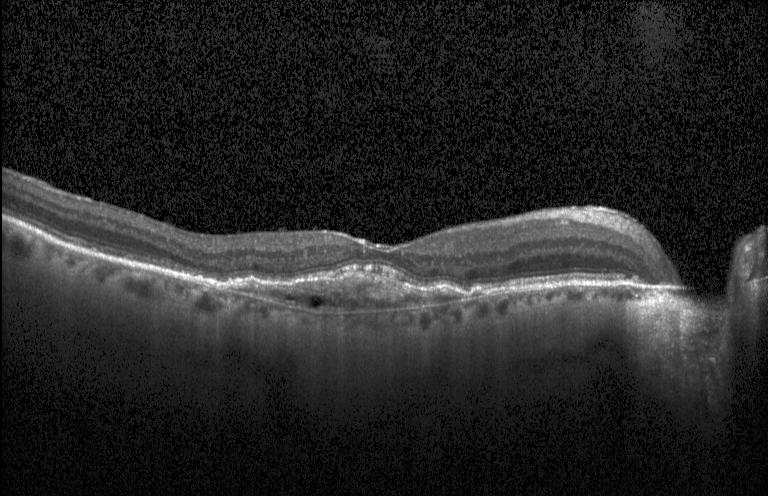 Finding: a choroidal neovascular membrane.